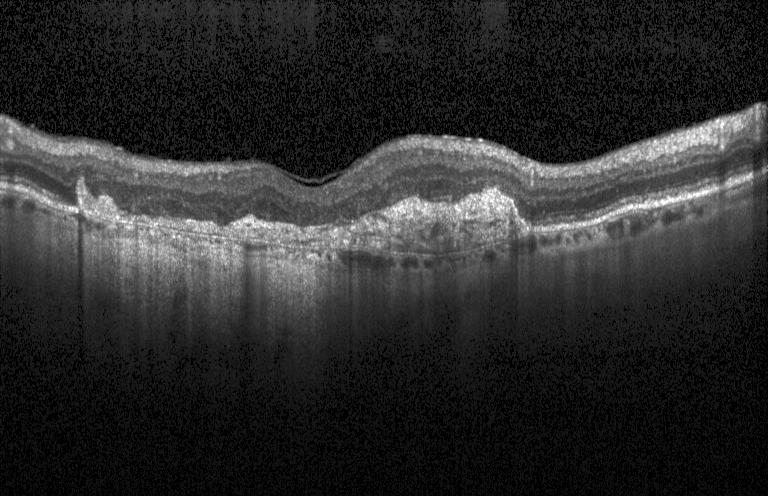
Retinal OCT B-scan, spectral-domain optical coherence tomography, macular scan
The scan shows choroidal neovascularization (CNV).